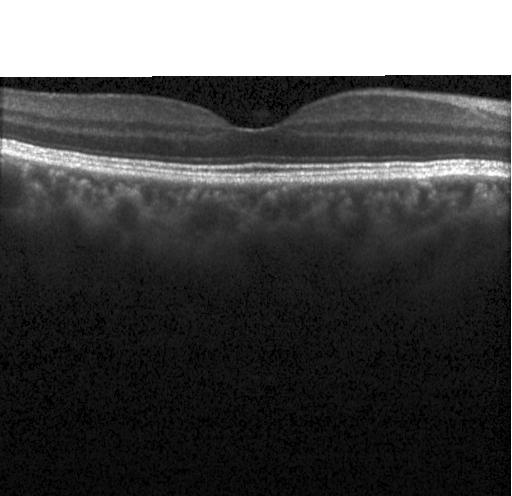
This B-scan demonstrates no choroidal neovascularization, no diabetic macular edema, and no drusen.